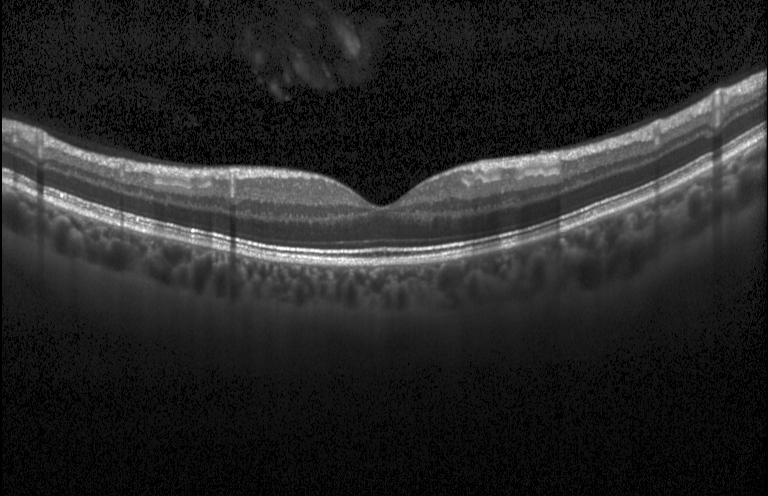
Retinal OCT B-scan — Impression: neither CNV, DME, nor drusen.